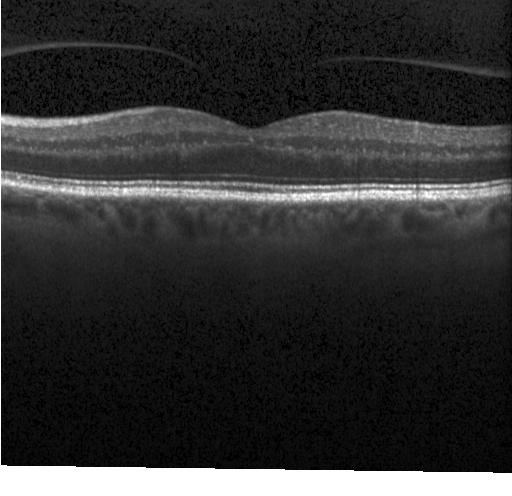
Diagnosis: no choroidal neovascularization, no diabetic macular edema, and no drusen.